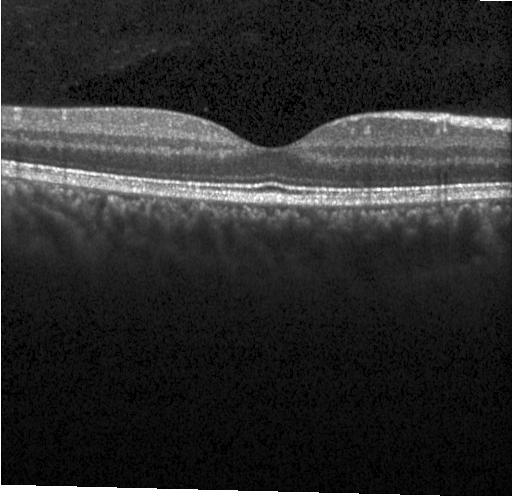

Impression: no choroidal neovascularization, diabetic macular edema, or drusen.